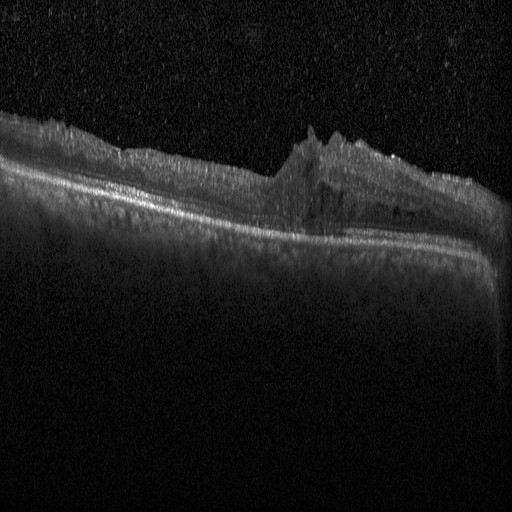

SD-OCT, horizontal scan through the fovea, instrument: Heidelberg Spectralis, optical coherence tomography scan. Finding: diabetic macular edema (DME).